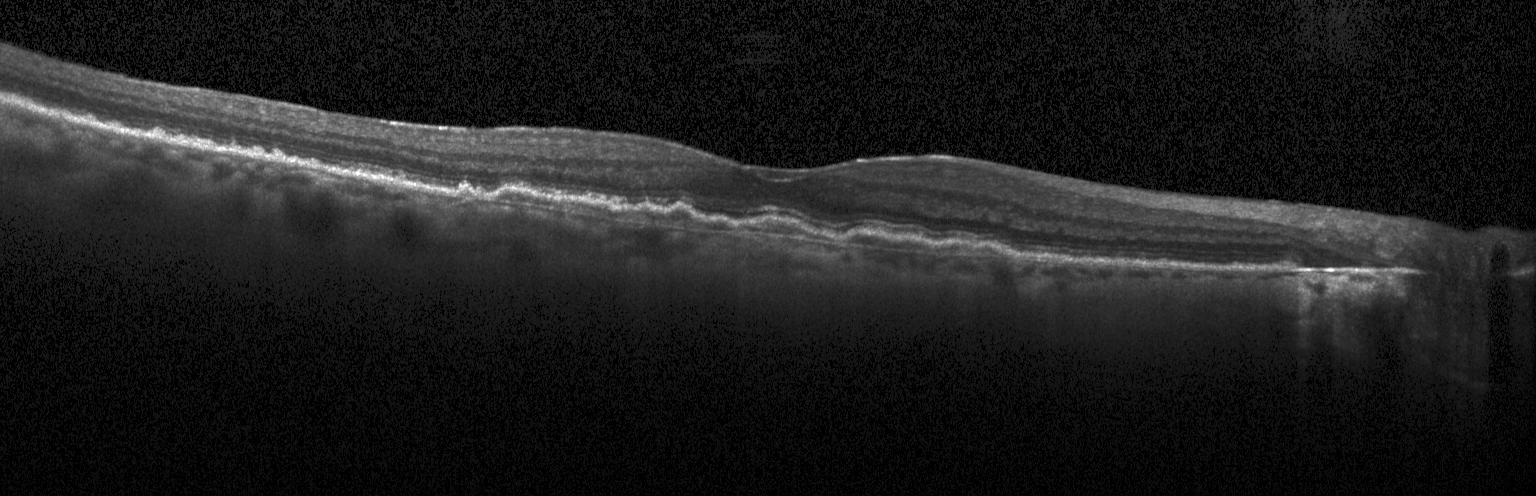

OCT finding: choroidal neovascularization (CNV).